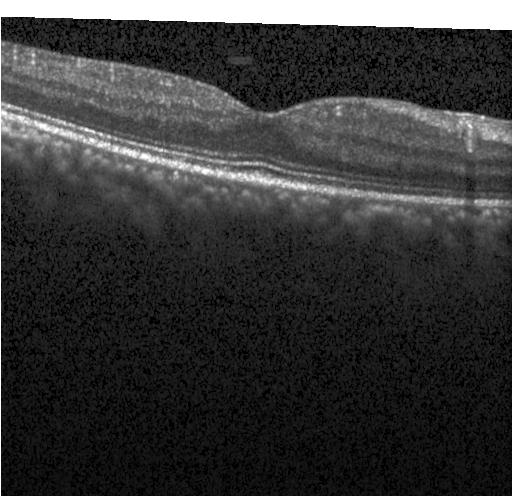
Macular OCT demonstrating no CNV, no DME, and no drusen.